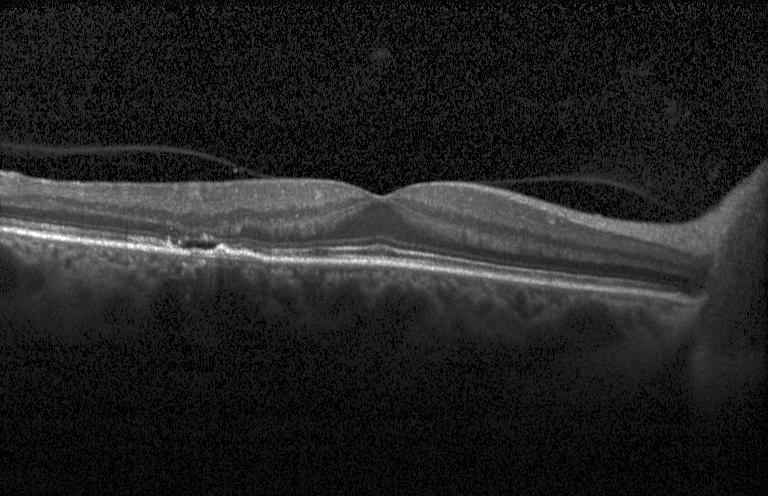

Diagnosis: choroidal neovascularization (CNV).